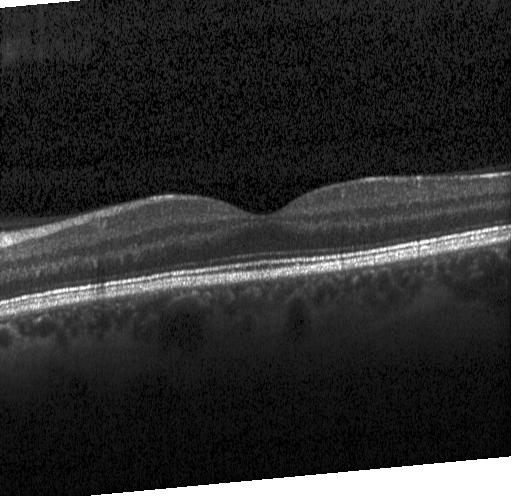
Diagnosis: neither choroidal neovascularization, diabetic macular edema, nor drusen.